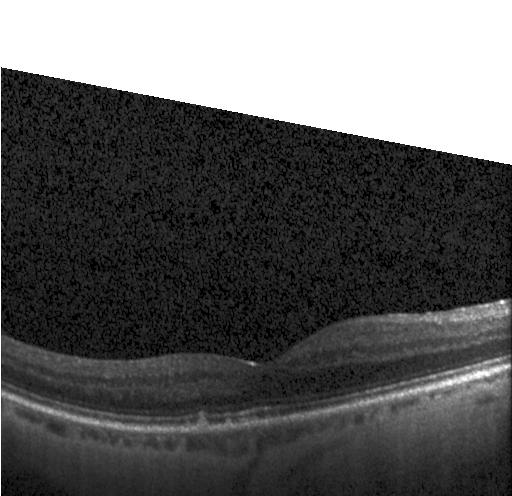
Spectral-domain OCT B-scan: drusen.